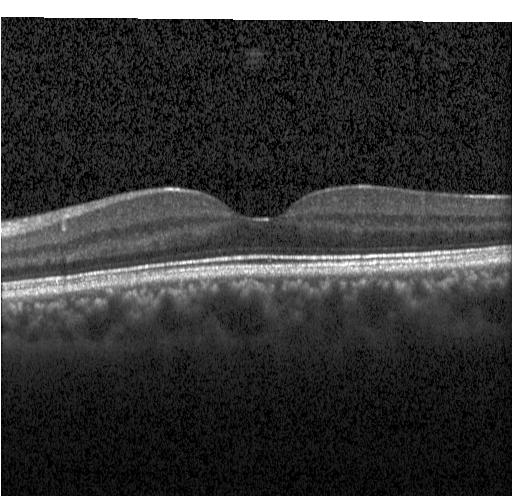

Macular OCT: no CNV, no DME, and no drusen.